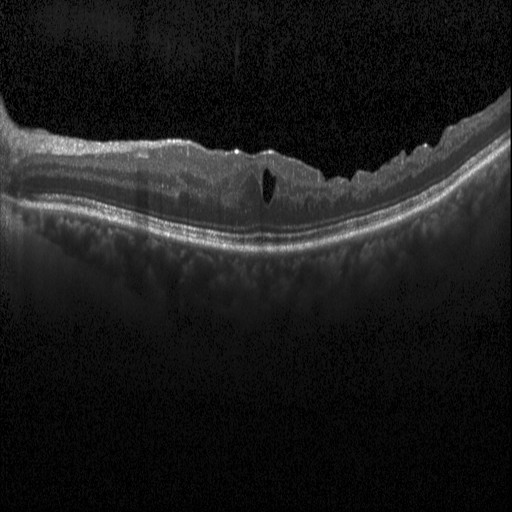
Spectral-domain optical coherence tomography; acquired on a Heidelberg Spectralis; optical coherence tomography scan
Assessment: diabetic macular edema (DME).